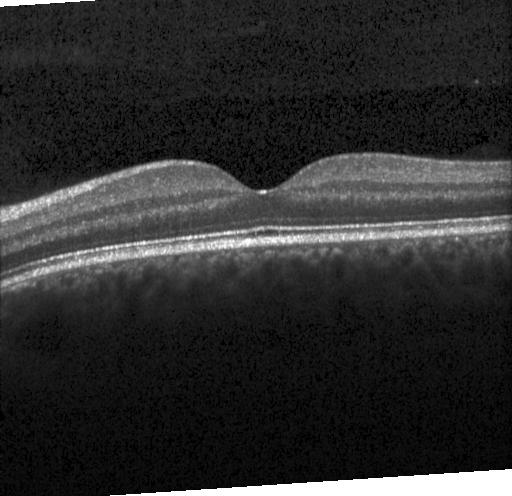

Finding: neither choroidal neovascularization, diabetic macular edema, nor drusen.